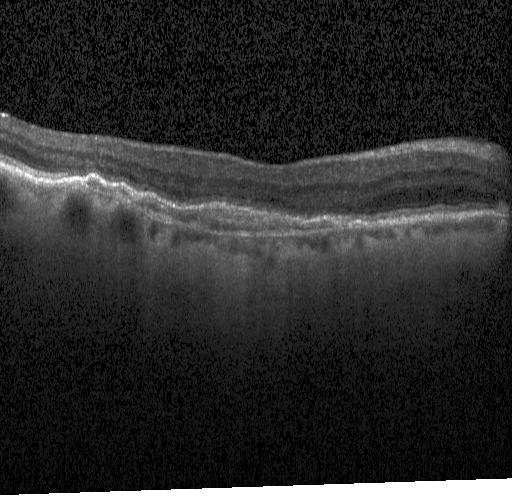 This B-scan demonstrates a choroidal neovascular membrane.